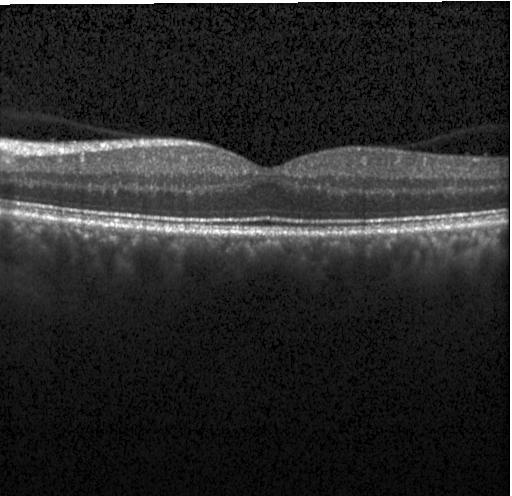 OCT scan showing no evidence of choroidal neovascularization, diabetic macular edema, or drusen.